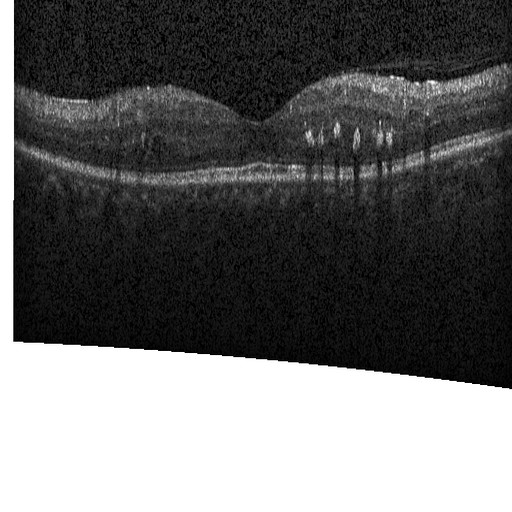 OCT B-scan showing DME.